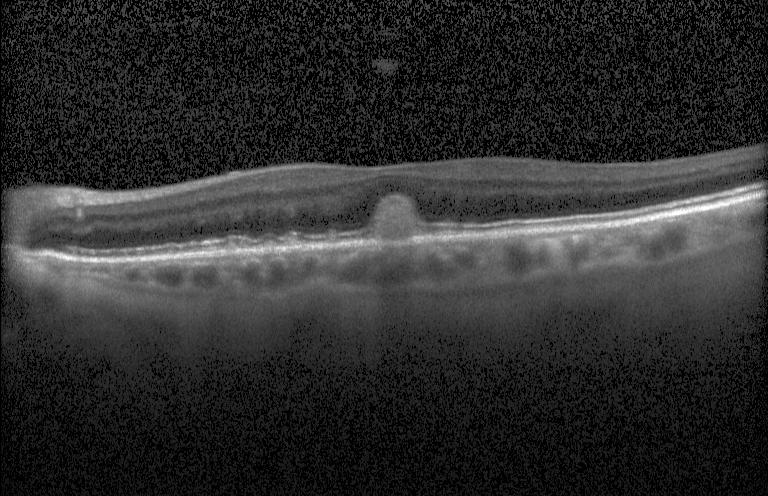 Spectral-domain OCT B-scan: a choroidal neovascular membrane.